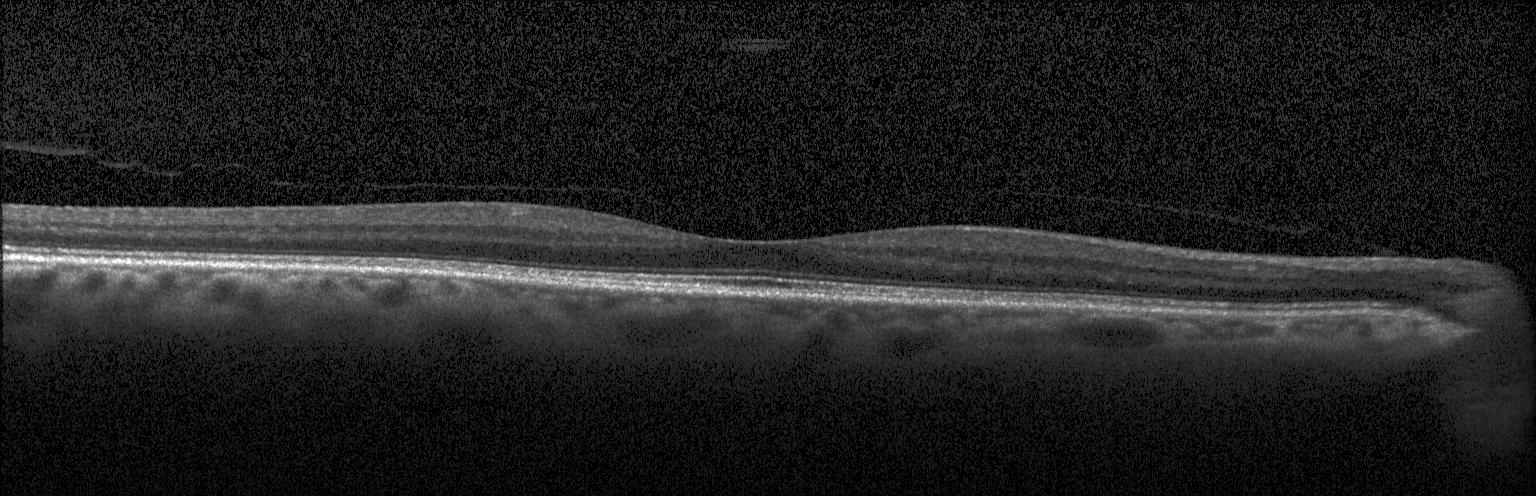 Heidelberg Spectralis OCT system, horizontal scan through the fovea, OCT line scan, SD-OCT. Macular OCT: no CNV, no DME, and no drusen.